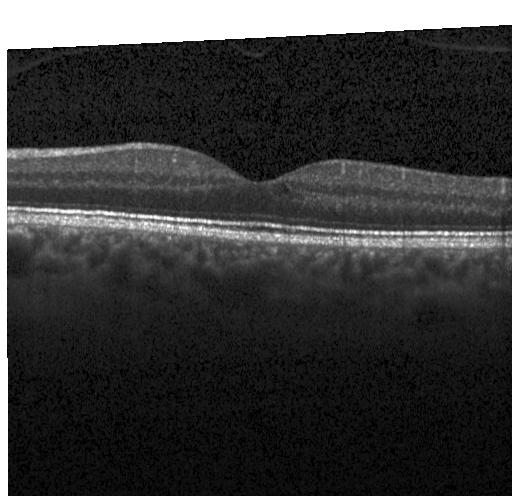

Impression: no evidence of CNV, DME, or drusen.